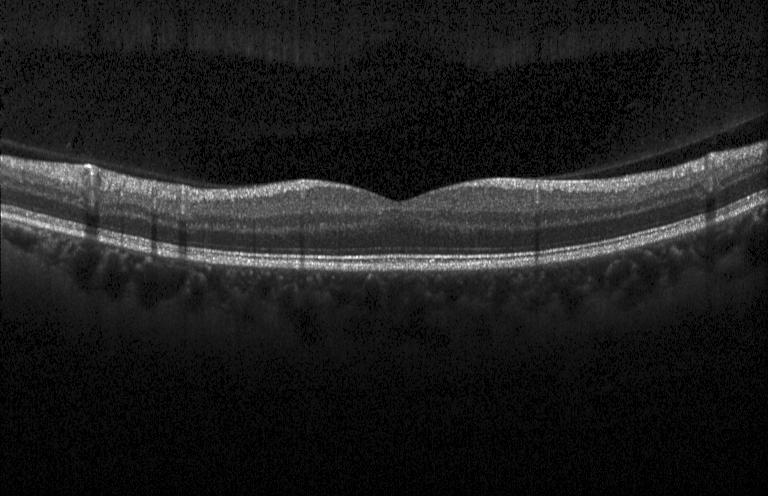 SD-OCT, instrument: Heidelberg Spectralis, OCT line scan — OCT finding: no choroidal neovascularization, diabetic macular edema, or drusen.